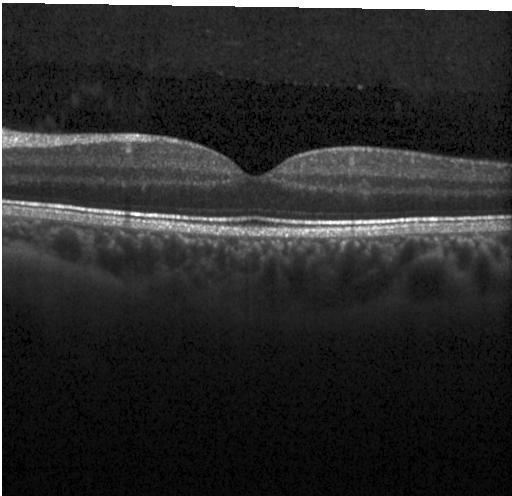

Diagnosis: neither CNV, DME, nor drusen.